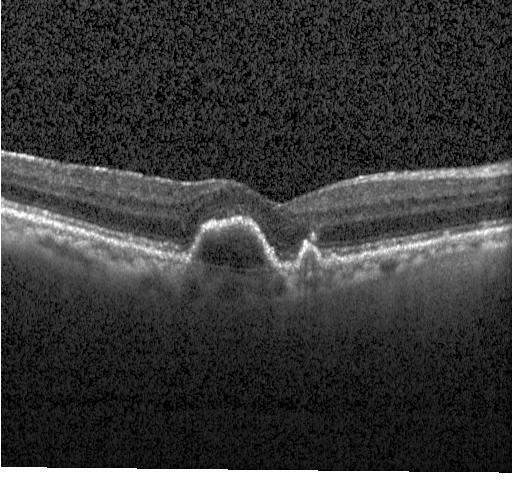

Optical coherence tomography scan; Heidelberg Spectralis OCT system
Finding: a choroidal neovascular membrane.